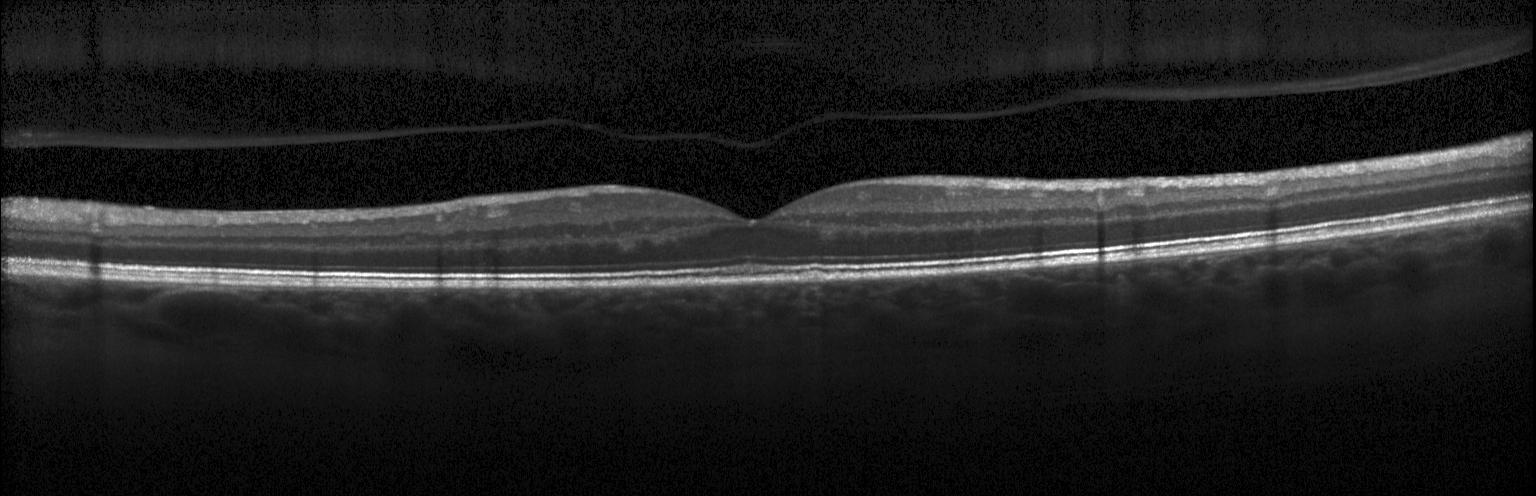

This B-scan demonstrates no evidence of choroidal neovascularization, diabetic macular edema, or drusen.